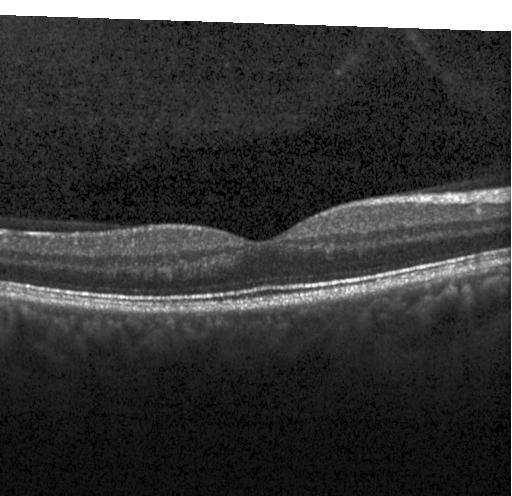
Macular OCT demonstrating no choroidal neovascularization, diabetic macular edema, or drusen.